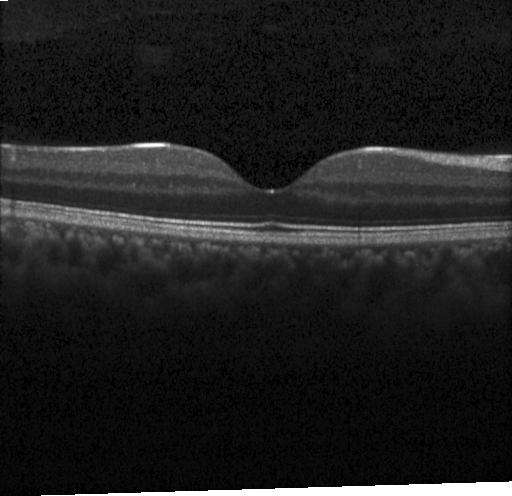 Finding: no evidence of choroidal neovascularization, diabetic macular edema, or drusen.